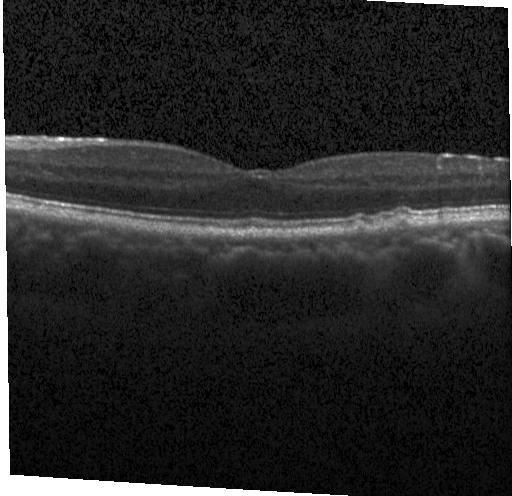
OCT scan showing multiple drusen.